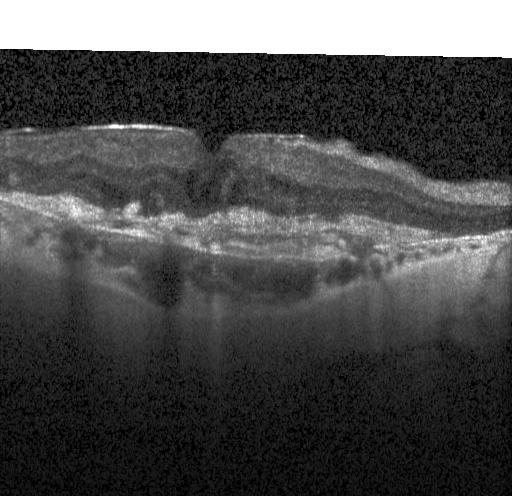 Macular OCT: a choroidal neovascular membrane.